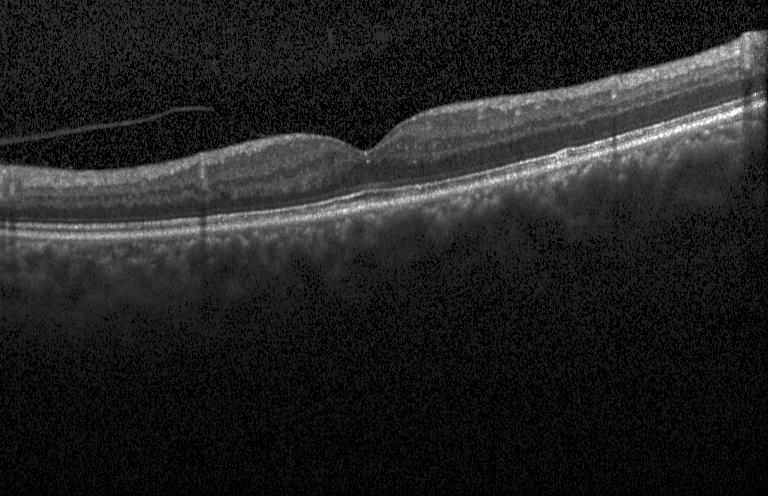 Finding: no CNV, no DME, and no drusen.